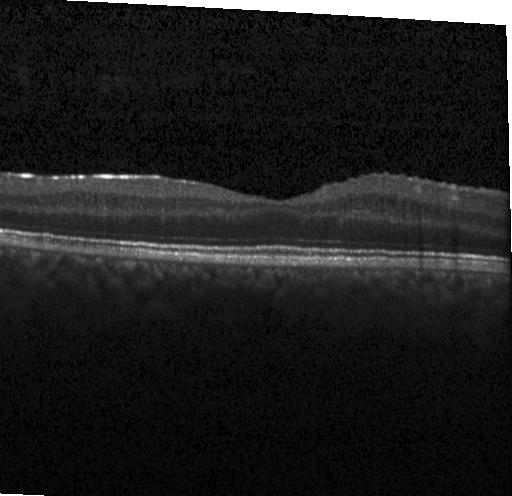

Spectral-domain optical coherence tomography · optical coherence tomography scan · centered on the fovea.
This B-scan demonstrates diabetic macular edema (DME).